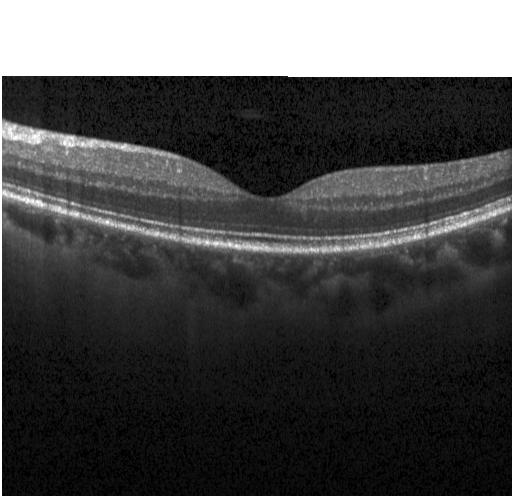
Optical coherence tomography scan, Heidelberg Spectralis OCT system. Impression: no evidence of CNV, DME, or drusen.